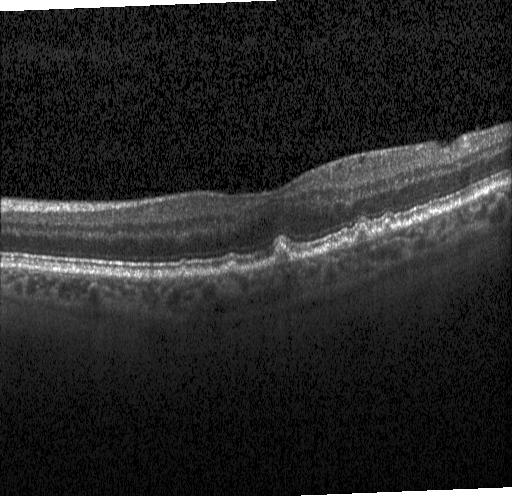
Diagnosis: sub-RPE drusenoid deposits.